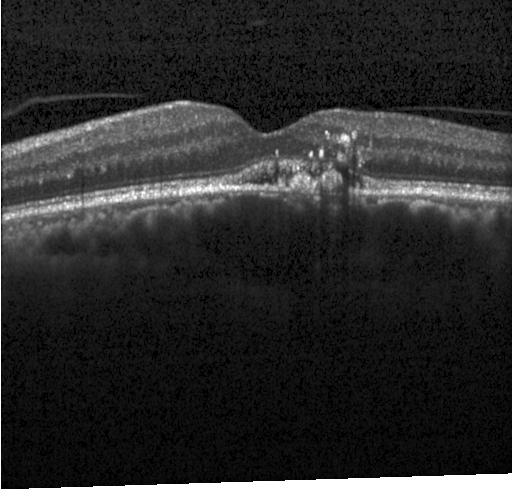

Macular OCT: a choroidal neovascular membrane.